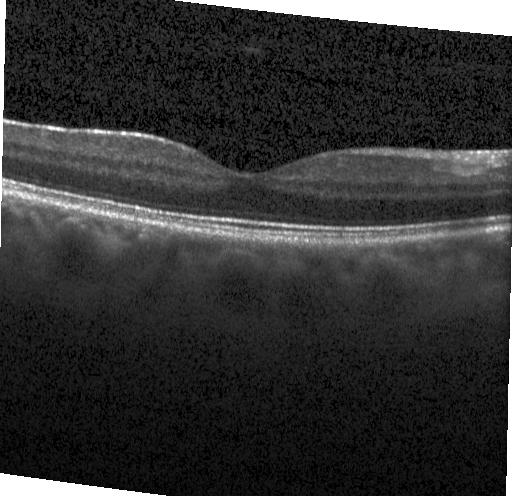 Optical coherence tomography B-scan, fovea-centered
No CNV, DME, or drusen.